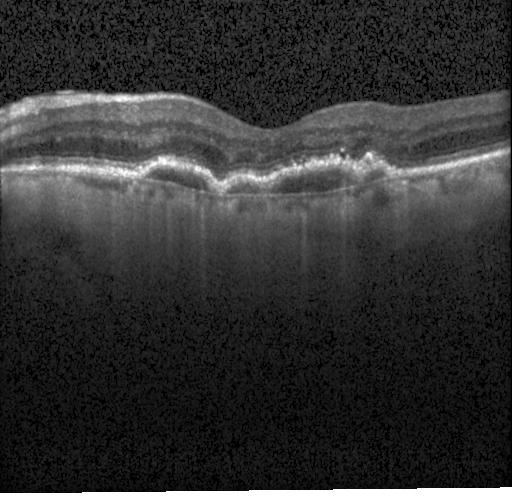 OCT B-scan. This B-scan demonstrates a choroidal neovascular membrane.